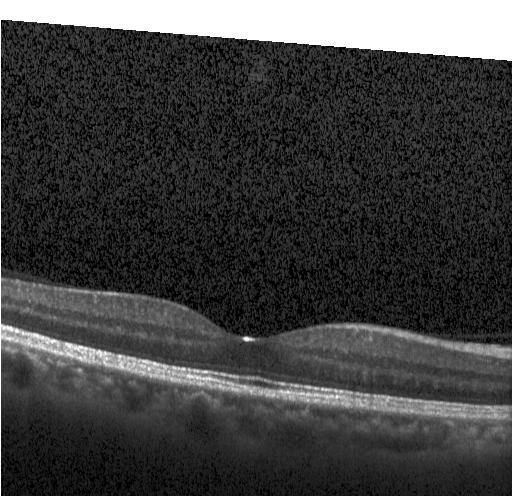

Horizontal scan through the fovea · retinal OCT cross-section — Impression: no CNV, DME, or drusen.